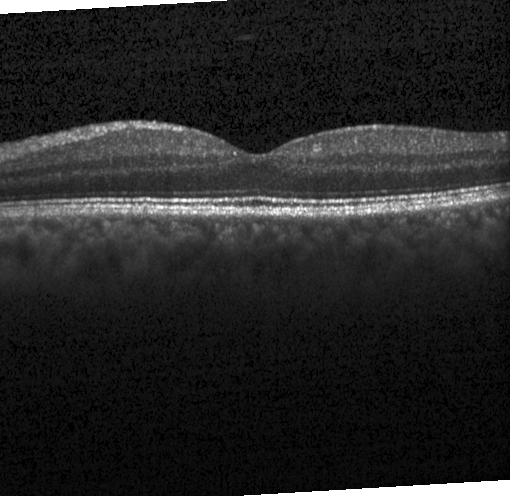

Dx: neither choroidal neovascularization, diabetic macular edema, nor drusen.